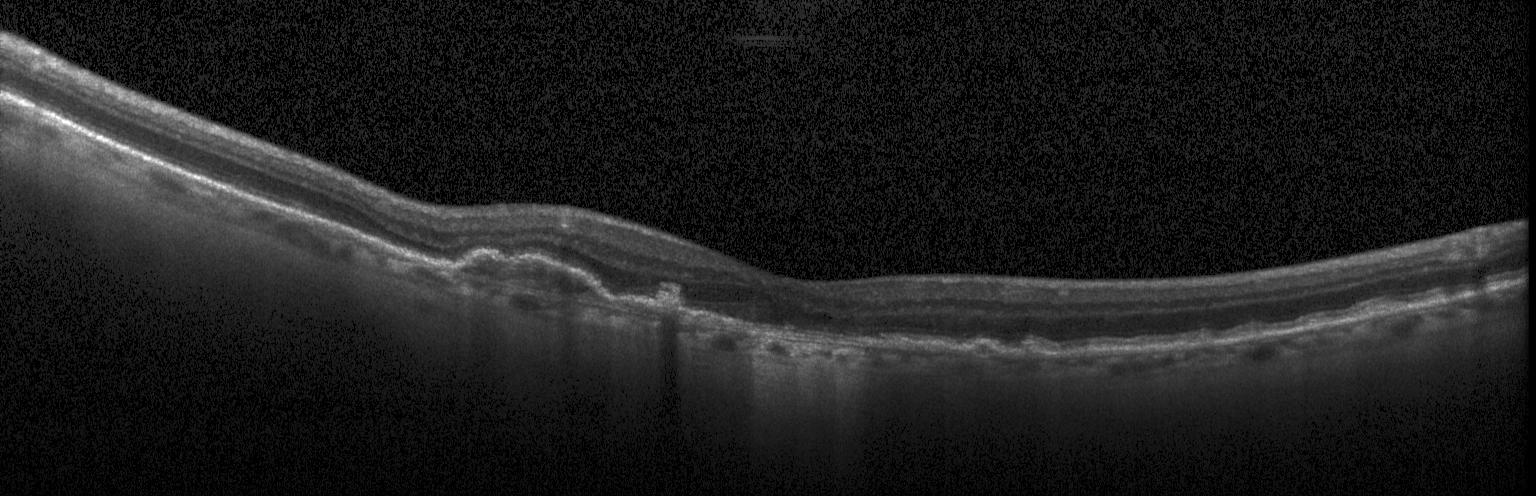 Macular OCT: choroidal neovascularization (CNV).